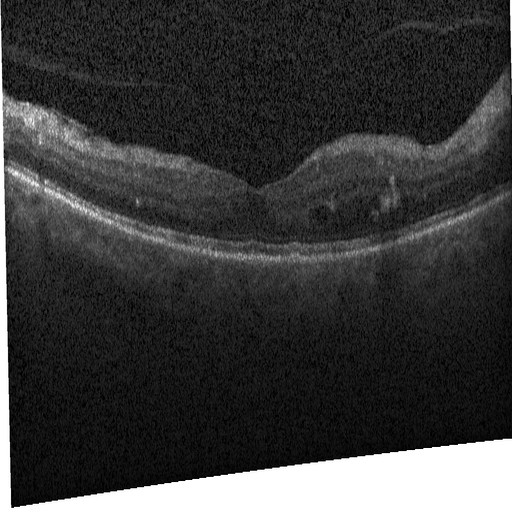 Diagnosis: diabetic macular edema (DME).